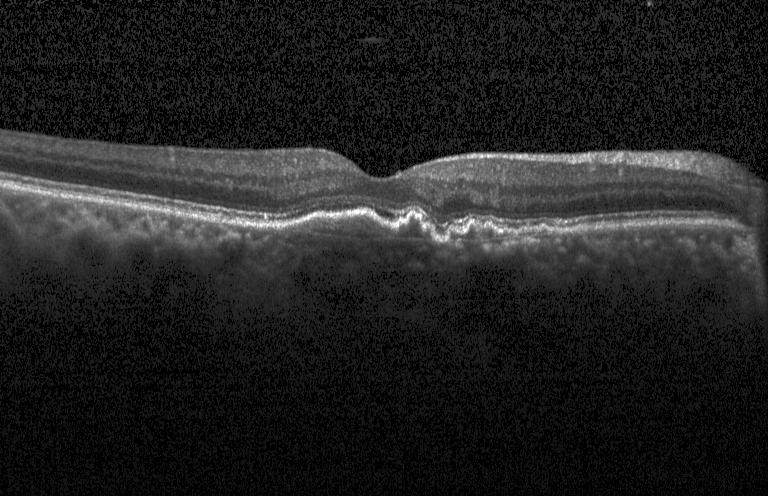

Retinal OCT cross-section · Heidelberg Spectralis. Drusen.